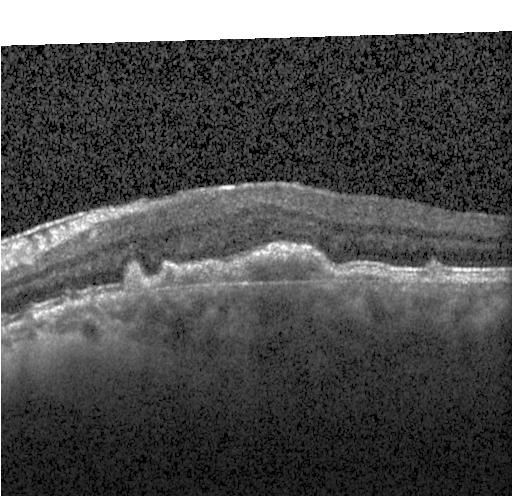
OCT line scan, SD-OCT — A choroidal neovascular membrane.